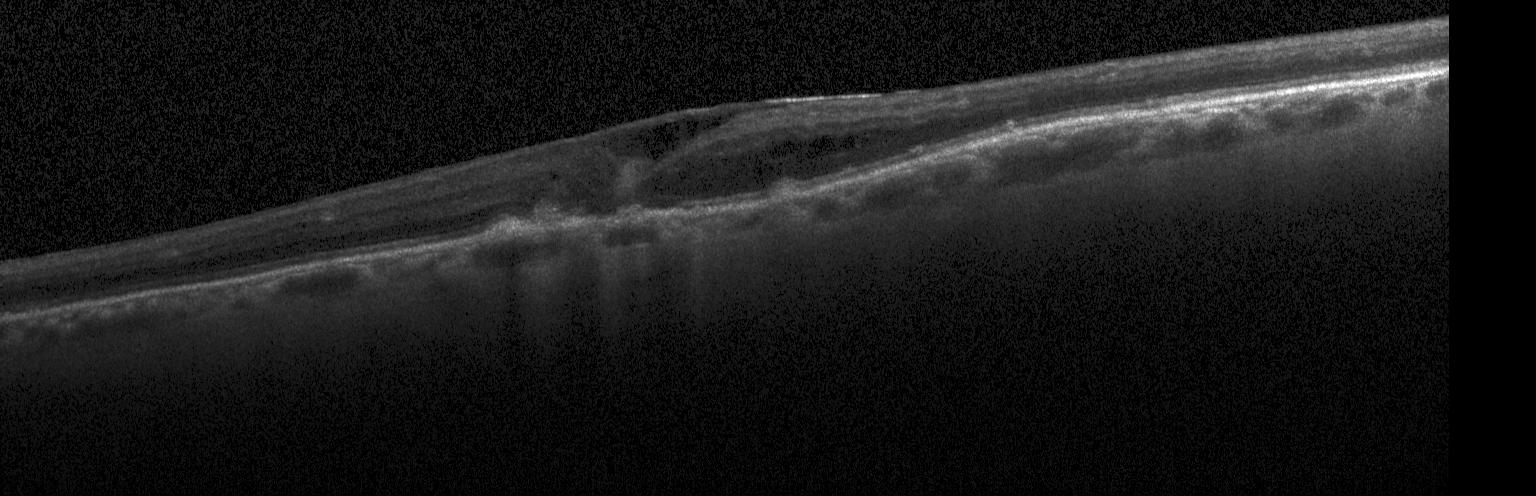

Optical coherence tomography B-scan; spectral-domain optical coherence tomography
Impression: choroidal neovascularization.